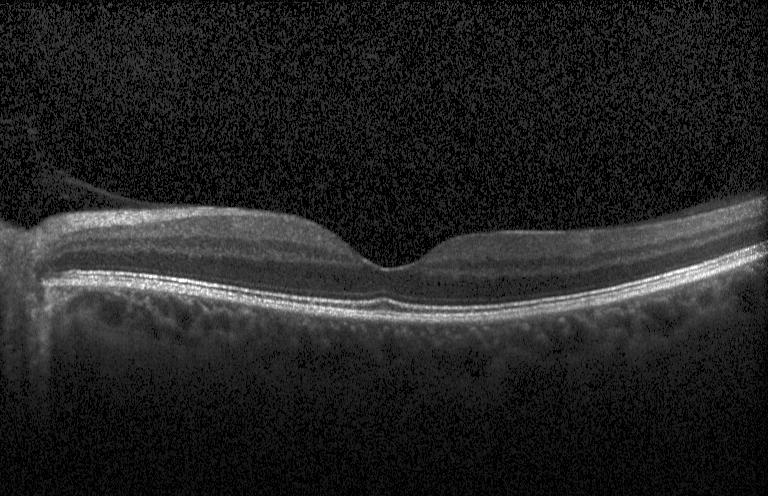 OCT finding: neither CNV, DME, nor drusen.